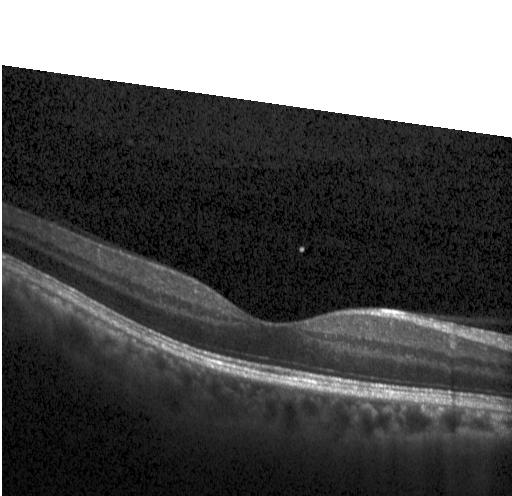

Retinal OCT B-scan. Diagnosis: no choroidal neovascularization, no diabetic macular edema, and no drusen.